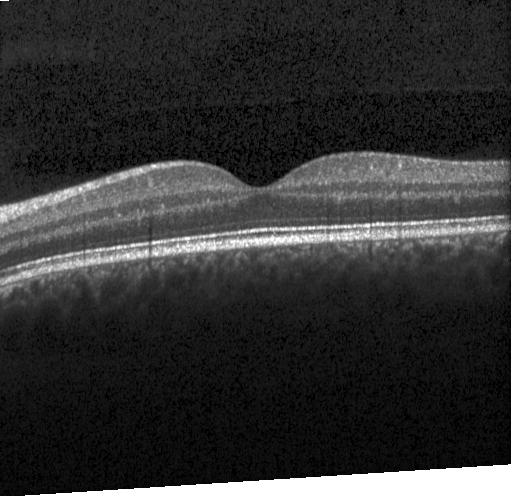

Centered on the fovea · optical coherence tomography scan
Impression: neither choroidal neovascularization, diabetic macular edema, nor drusen.